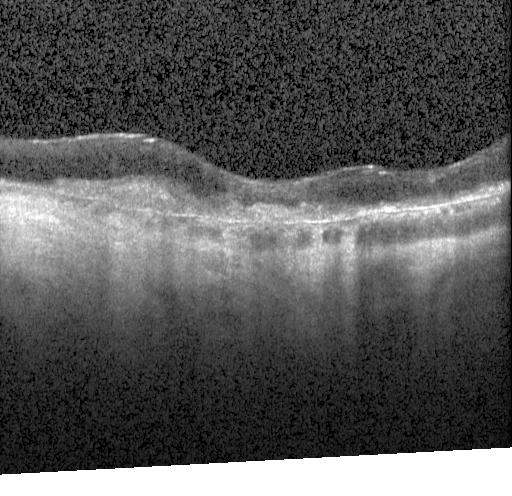 OCT B-scan; spectral-domain optical coherence tomography — Impression: CNV.